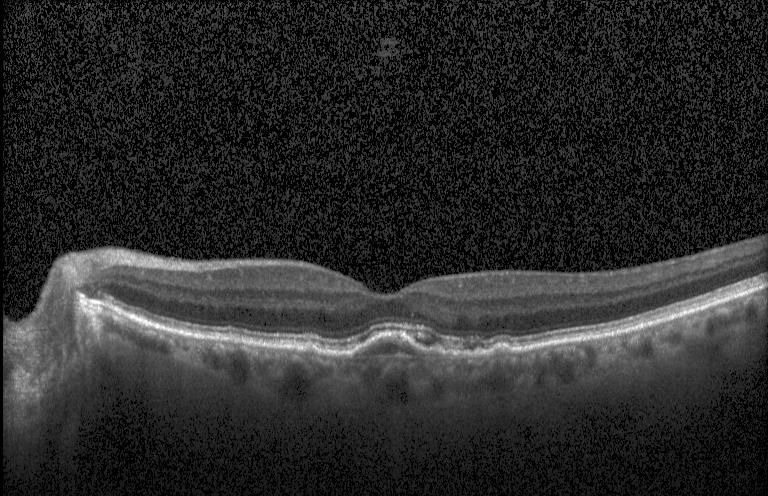 Heidelberg Spectralis, retinal OCT cross-section. Macular OCT: choroidal neovascularization (CNV).